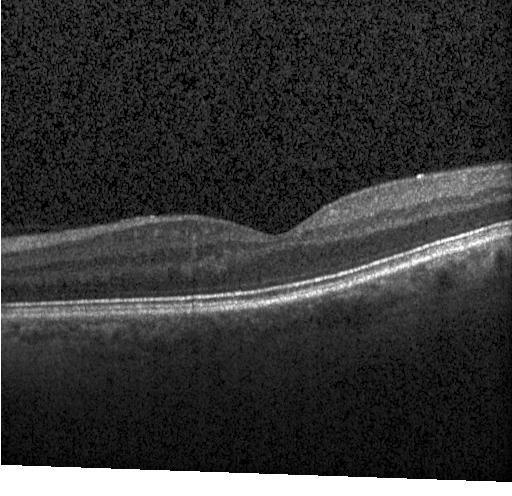
Diagnosis: no evidence of choroidal neovascularization, diabetic macular edema, or drusen.